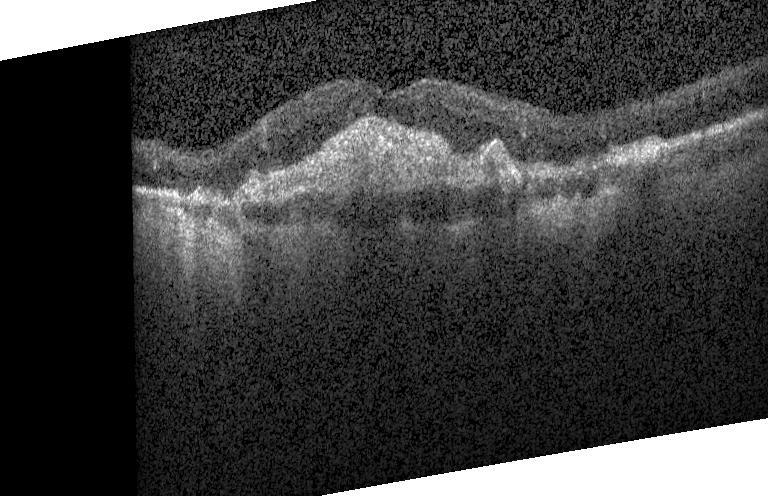
OCT B-scan.
Diagnosis: a choroidal neovascular membrane.